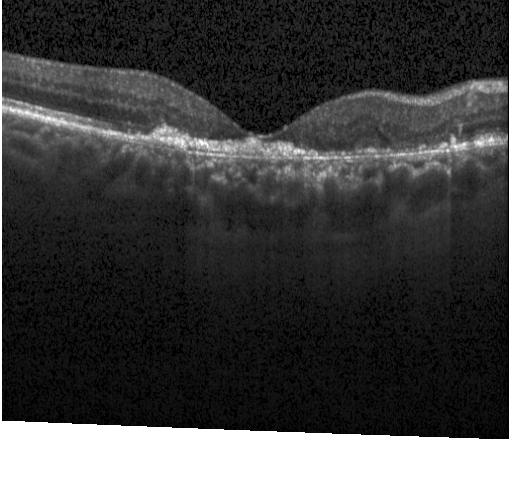

Finding: choroidal neovascularization (CNV).